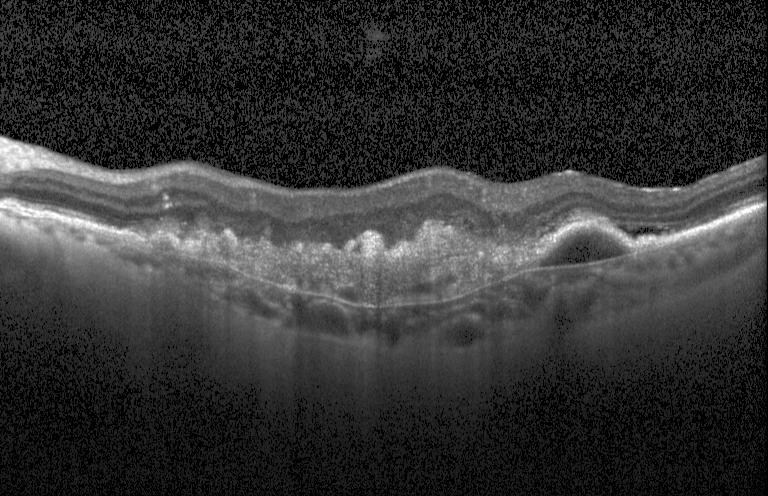

Centered on the fovea, spectral-domain OCT, optical coherence tomography scan, Heidelberg Spectralis. Assessment: CNV.